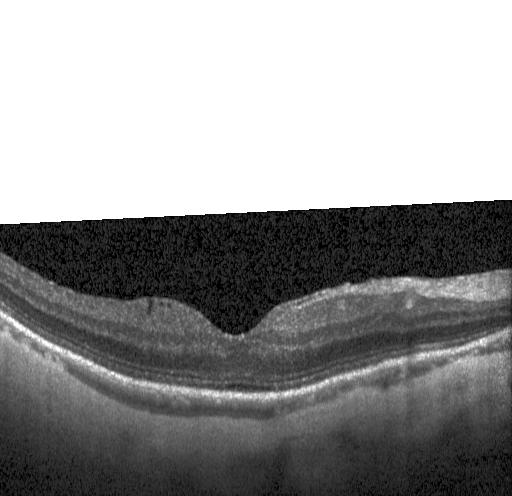

Centered on the fovea. Spectral-domain OCT. Heidelberg Spectralis. Optical coherence tomography scan — Assessment: neither choroidal neovascularization, diabetic macular edema, nor drusen.